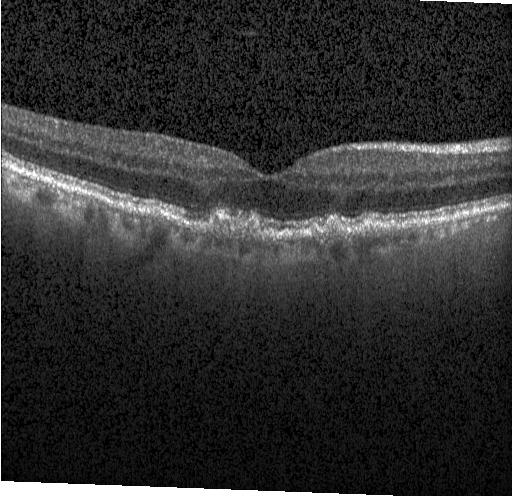

Retinal OCT cross-section showing sub-RPE drusenoid deposits.